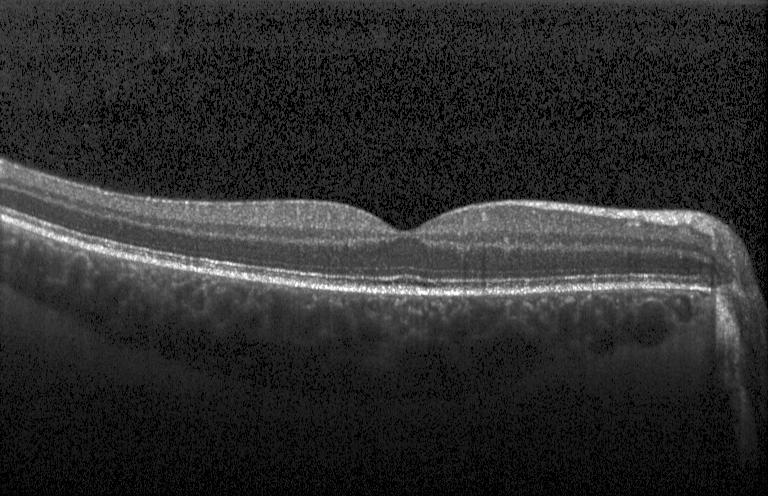

Macular OCT demonstrating no evidence of CNV, DME, or drusen.